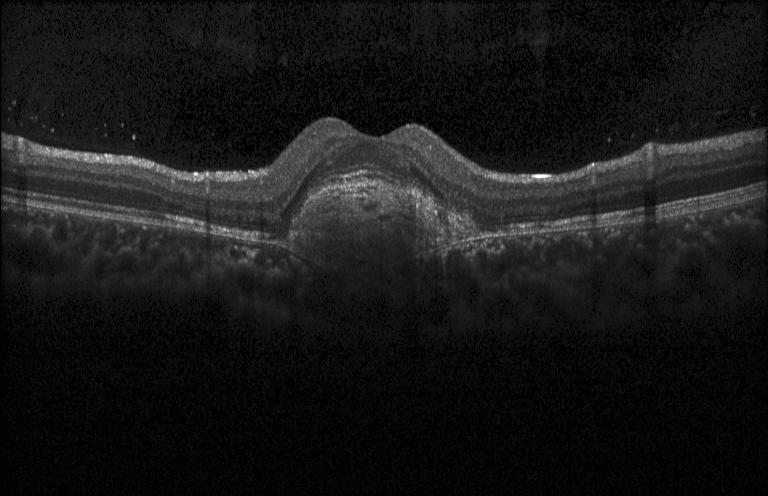 Macular OCT: a choroidal neovascular membrane.